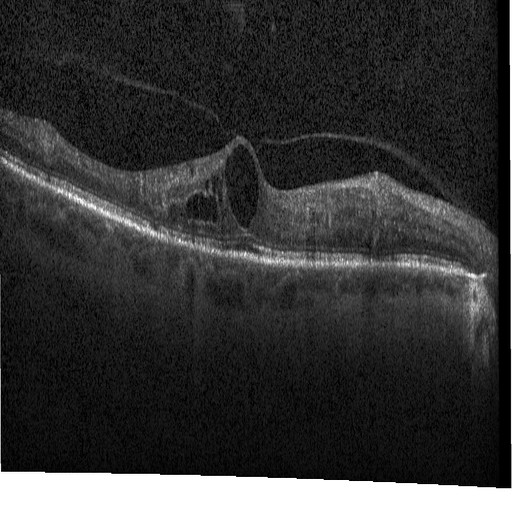

Spectral-domain OCT · retinal OCT B-scan. Macular OCT: diabetic macular edema (DME).